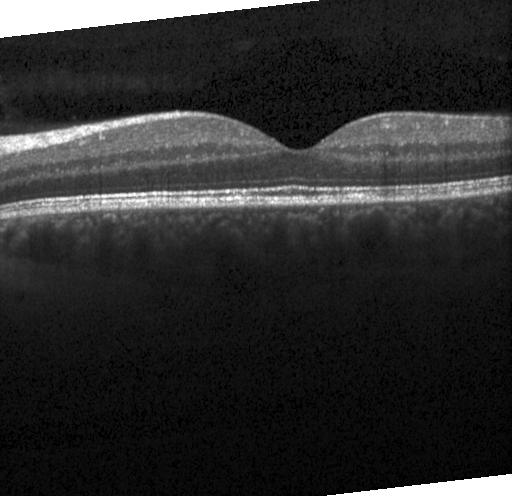

OCT B-scan. Heidelberg Spectralis OCT system. Centered on the fovea. Spectral-domain OCT. Diagnosis: no evidence of choroidal neovascularization, diabetic macular edema, or drusen.